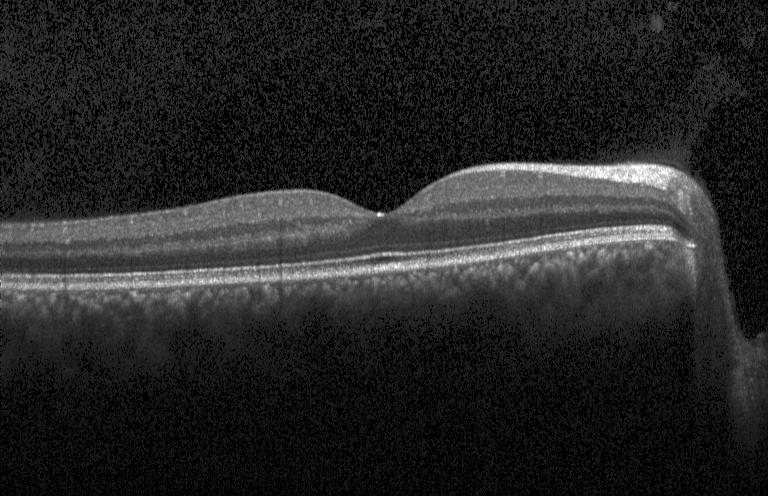

SD-OCT, OCT B-scan
This B-scan demonstrates no CNV, no DME, and no drusen.